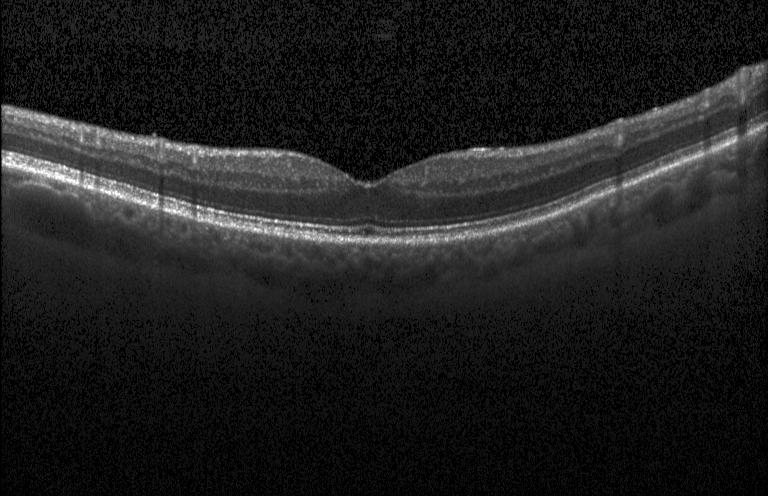
Impression: neither choroidal neovascularization, diabetic macular edema, nor drusen.